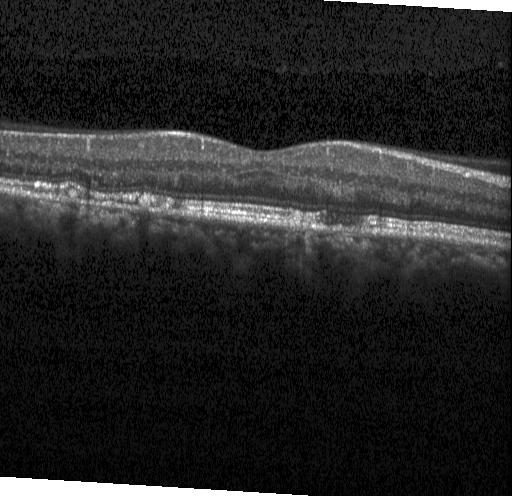 Retinal OCT cross-section, instrument: Heidelberg Spectralis. The scan shows drusen.